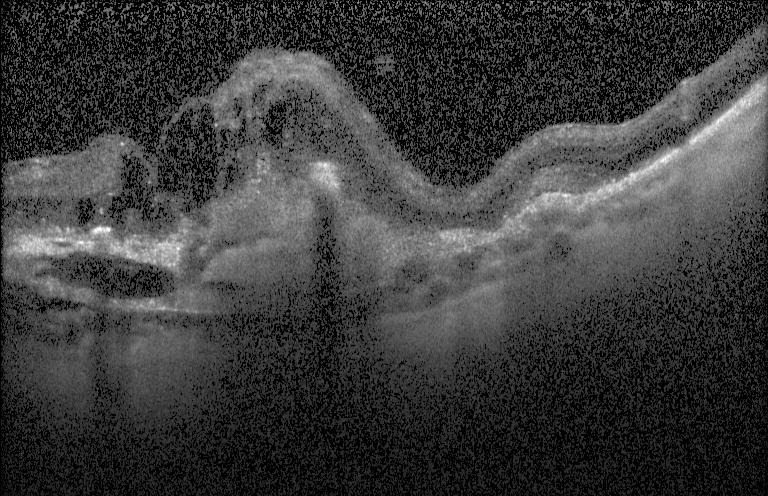
Spectral-domain OCT; centered on the fovea; retinal OCT cross-section.
This B-scan demonstrates a choroidal neovascular membrane.